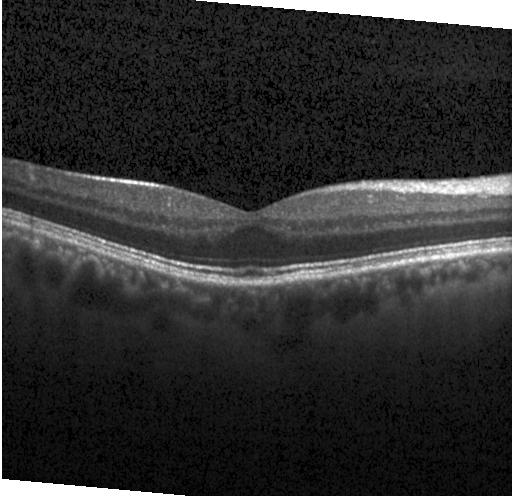

Finding: no choroidal neovascularization, diabetic macular edema, or drusen.